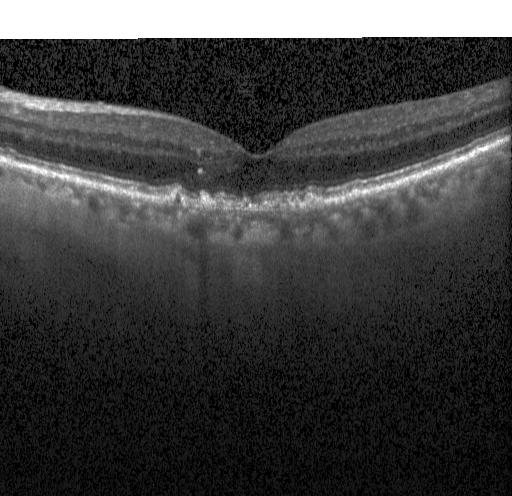

Instrument: Heidelberg Spectralis, macular scan, optical coherence tomography scan, spectral-domain OCT — Macular OCT: multiple drusen.